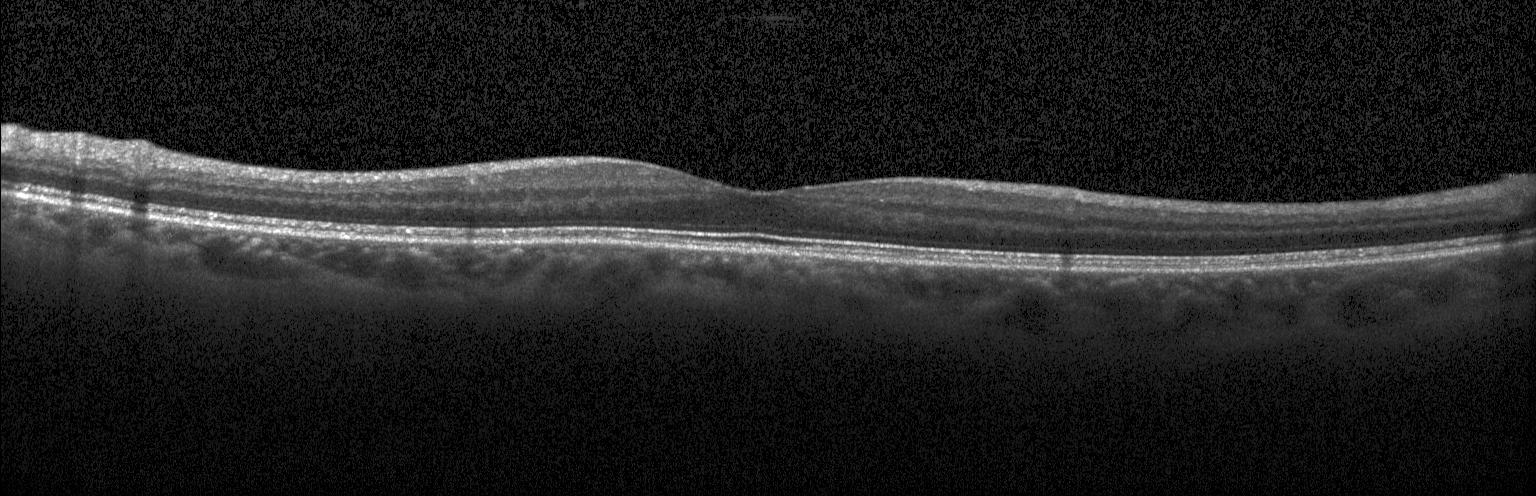
Optical coherence tomography B-scan. SD-OCT — Impression: no evidence of choroidal neovascularization, diabetic macular edema, or drusen.